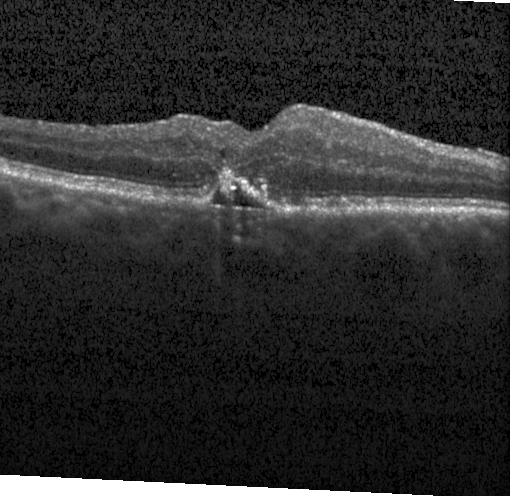

Spectral-domain optical coherence tomography. OCT B-scan. Fovea-centered. Acquired on a Heidelberg Spectralis. Impression: CNV.